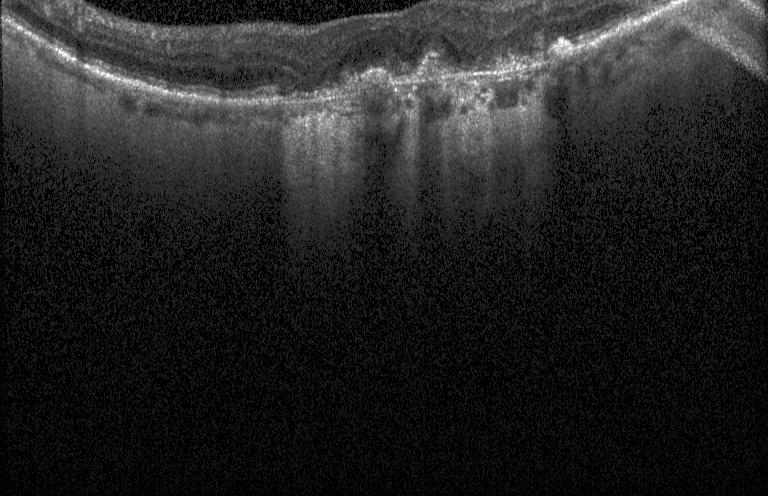
Impression: a choroidal neovascular membrane.